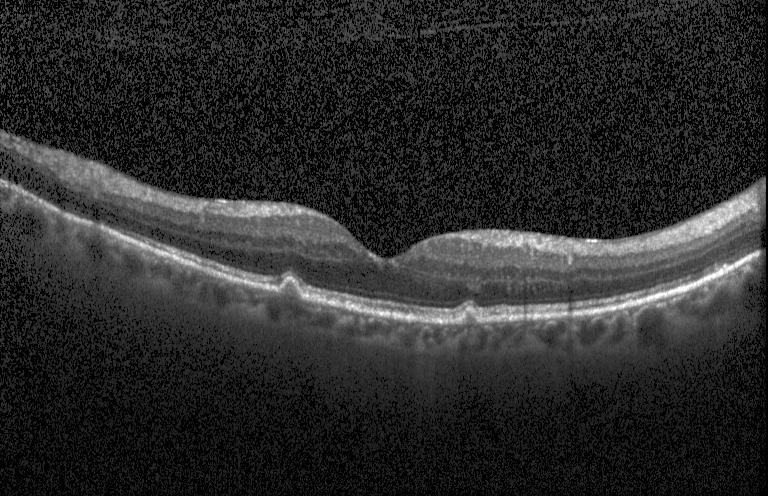

Macular OCT: multiple drusen.